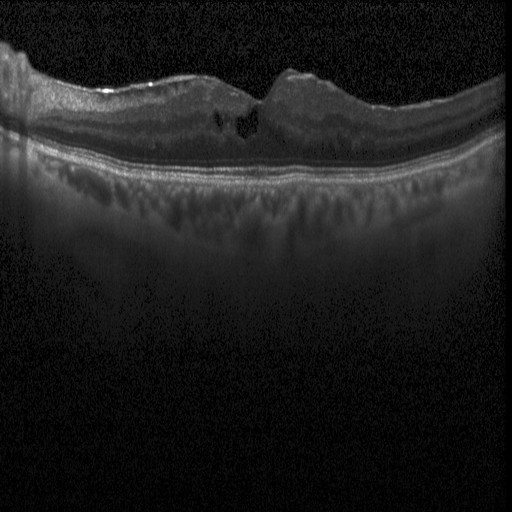

Spectral-domain OCT B-scan: diabetic macular edema (DME).